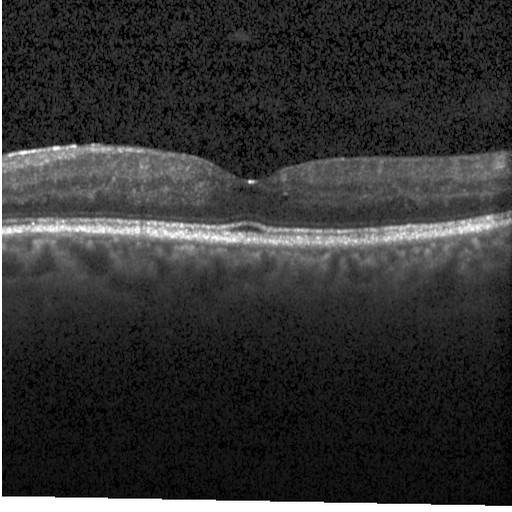
Instrument: Heidelberg Spectralis. Macular scan. Optical coherence tomography B-scan. Spectral-domain OCT. OCT finding: DME.